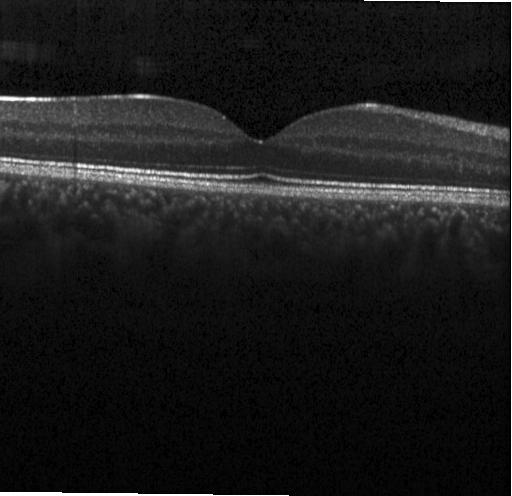
Instrument: Heidelberg Spectralis · fovea-centered · retinal OCT B-scan
Macular OCT: neither choroidal neovascularization, diabetic macular edema, nor drusen.